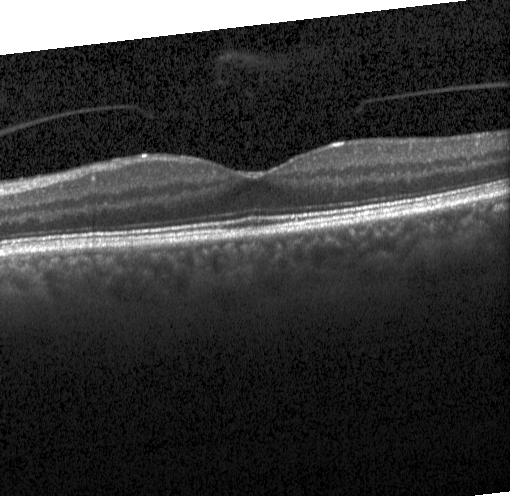

Spectral-domain optical coherence tomography; optical coherence tomography B-scan; Heidelberg Spectralis; horizontal scan through the fovea.
Finding: neither CNV, DME, nor drusen.